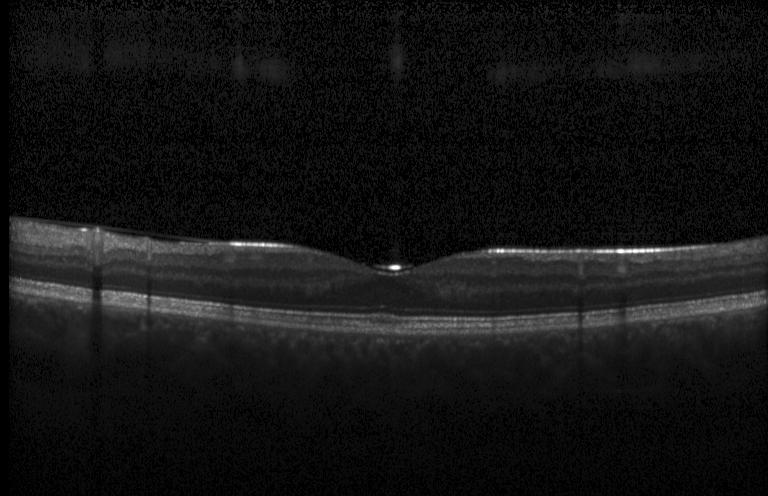 Retinal OCT cross-section; fovea-centered — Impression: no evidence of choroidal neovascularization, diabetic macular edema, or drusen.